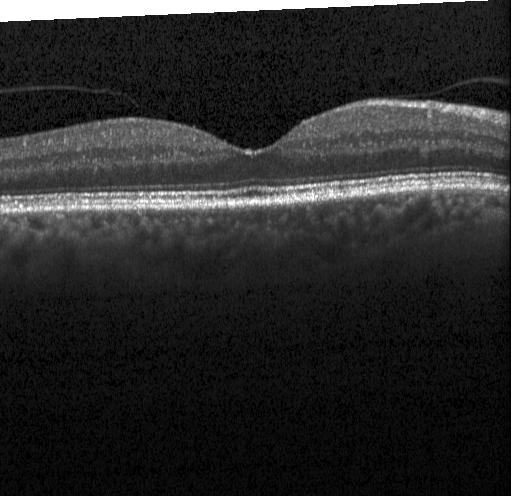

Retinal OCT cross-section
The scan shows no evidence of CNV, DME, or drusen.